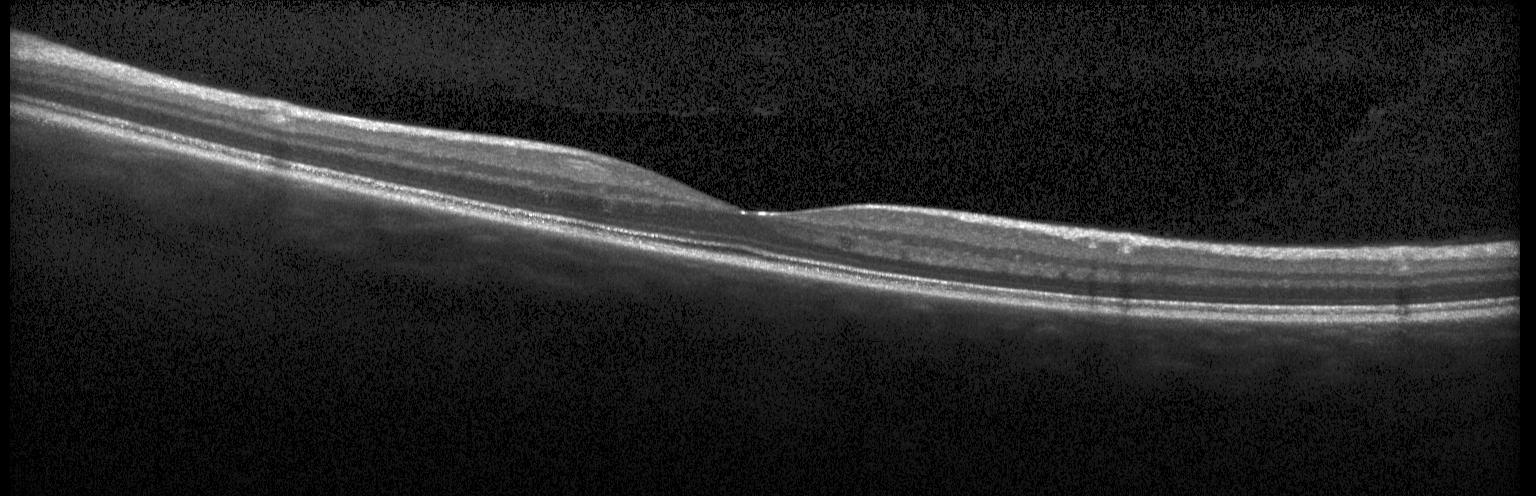 OCT scan showing no choroidal neovascularization, diabetic macular edema, or drusen.